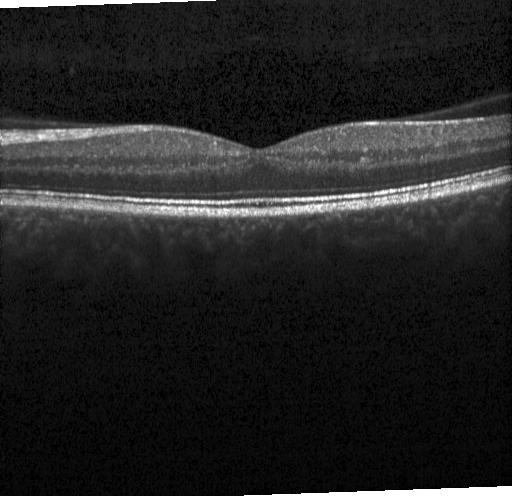
Retinal OCT B-scan. Impression: no choroidal neovascularization, diabetic macular edema, or drusen.